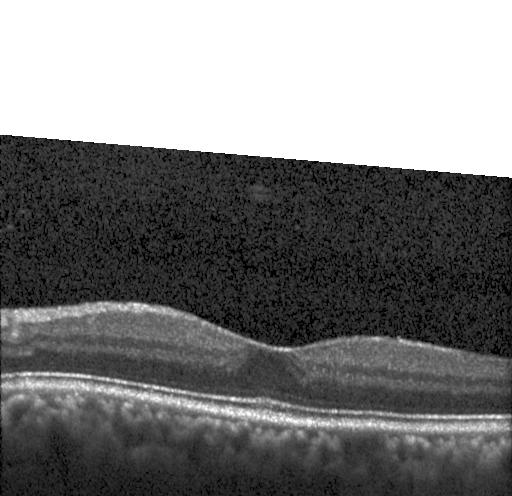
Diagnosis: neither choroidal neovascularization, diabetic macular edema, nor drusen.